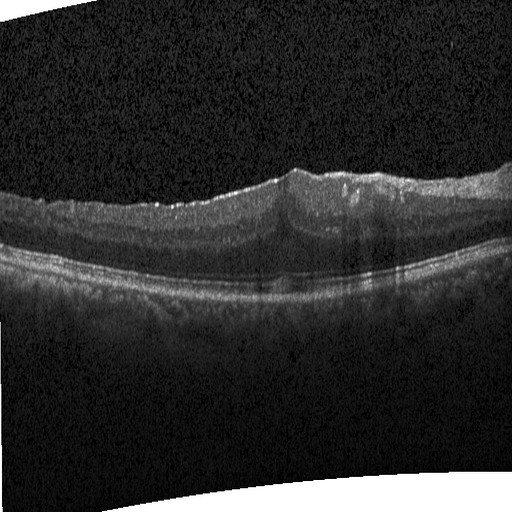

Retinal OCT cross-section
Assessment: DME.